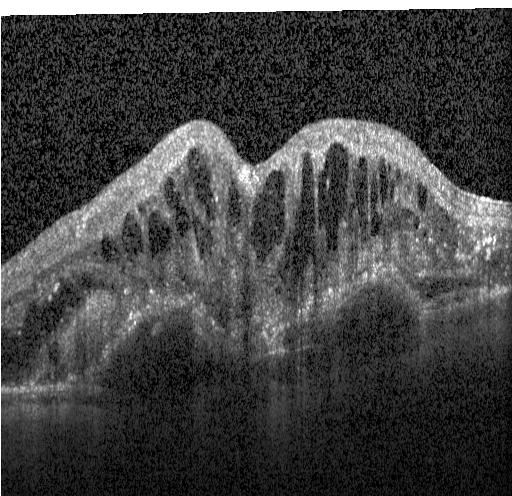
Impression: a choroidal neovascular membrane.